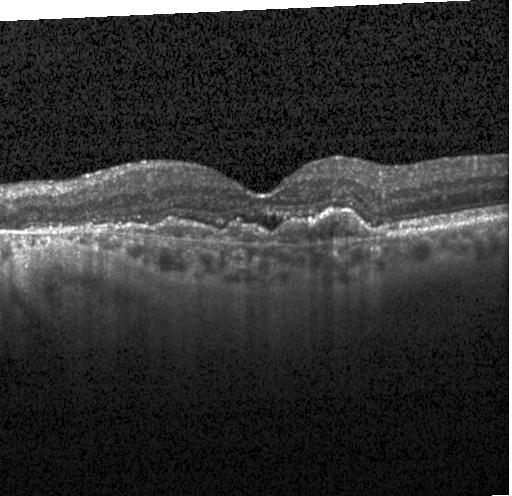

OCT scan showing a choroidal neovascular membrane.